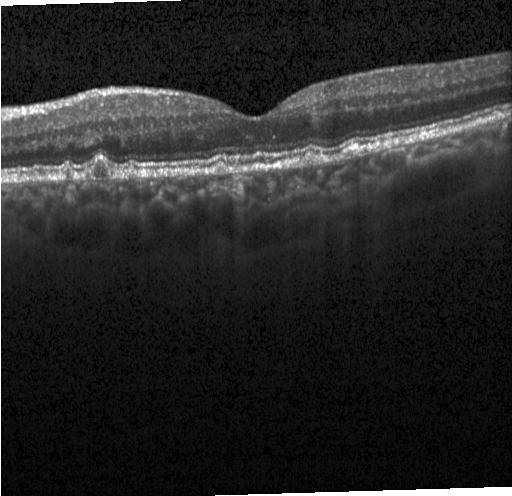 Retinal OCT B-scan. Spectral-domain OCT. Centered on the fovea. Acquired on a Heidelberg Spectralis. Finding: sub-RPE drusenoid deposits.